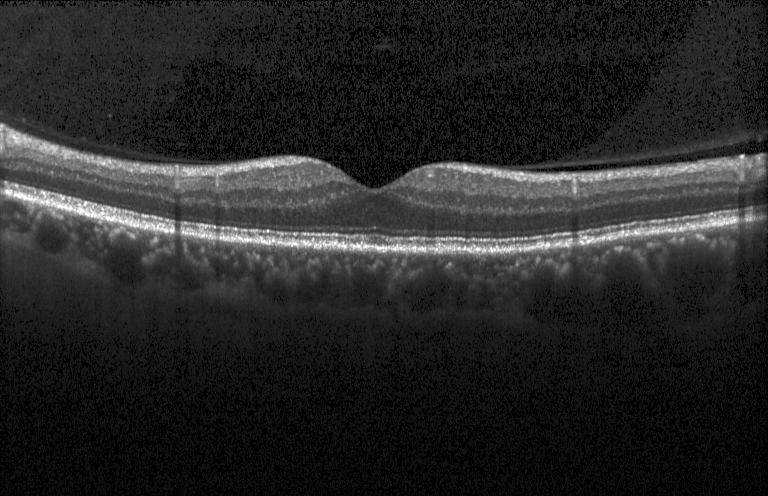 Retinal OCT cross-section; Heidelberg Spectralis OCT system.
Finding: no choroidal neovascularization, no diabetic macular edema, and no drusen.